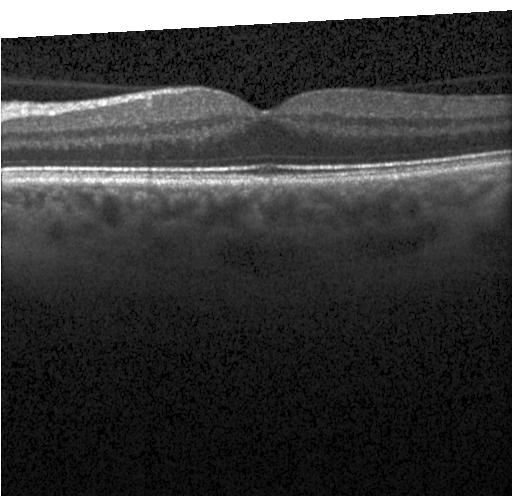
Through the macula, retinal OCT cross-section
Impression: no evidence of choroidal neovascularization, diabetic macular edema, or drusen.